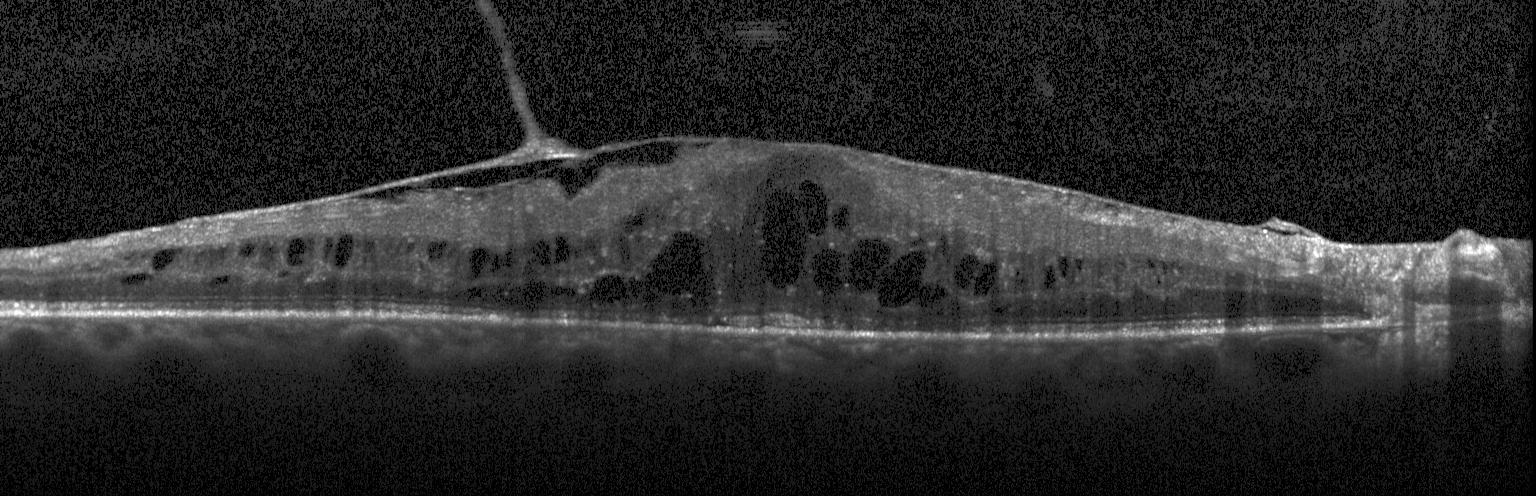
Spectral-domain OCT. OCT B-scan.
Impression: diabetic macular edema (DME).